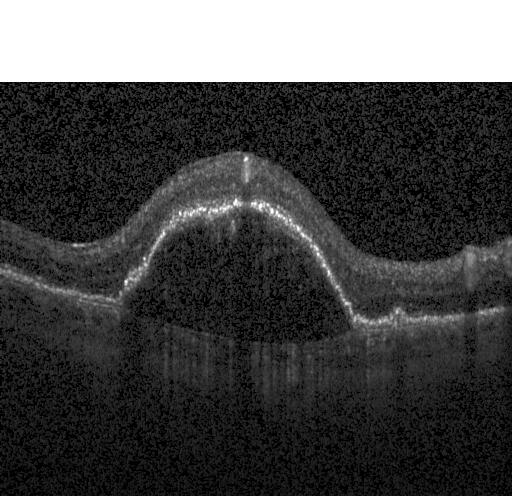 Spectral-domain OCT B-scan: a choroidal neovascular membrane.